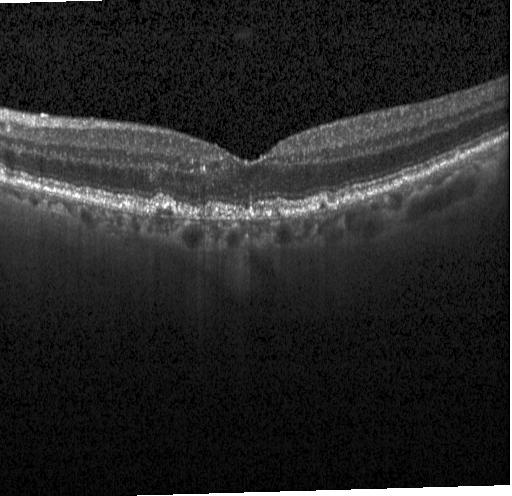 Multiple drusen.